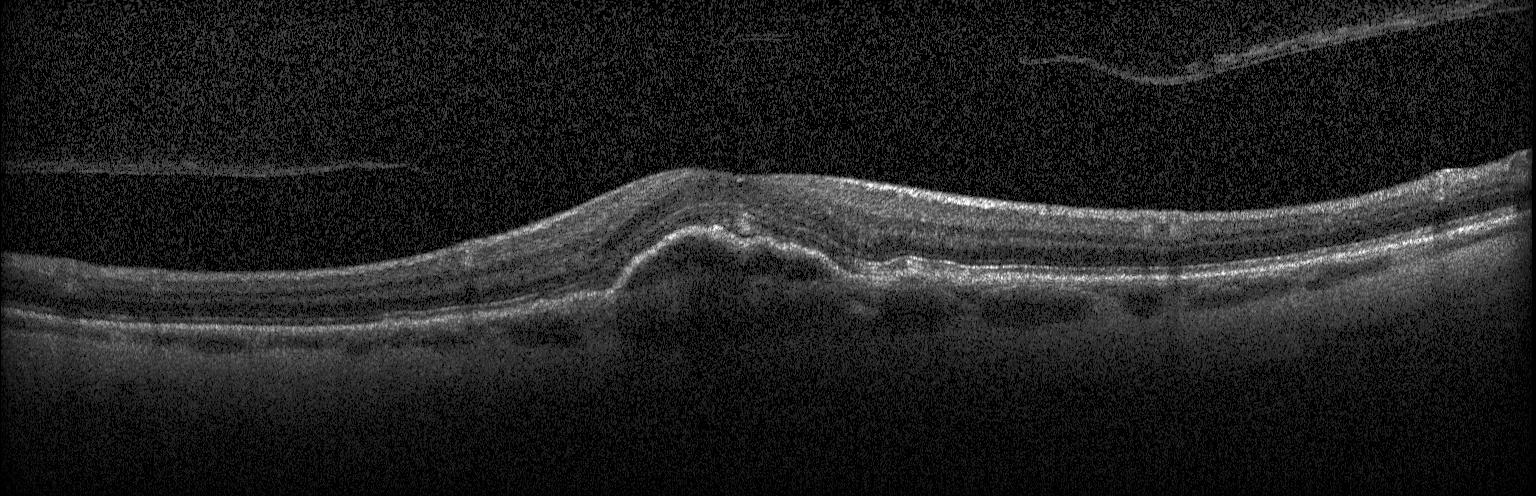
Retinal OCT cross-section. Finding: CNV.